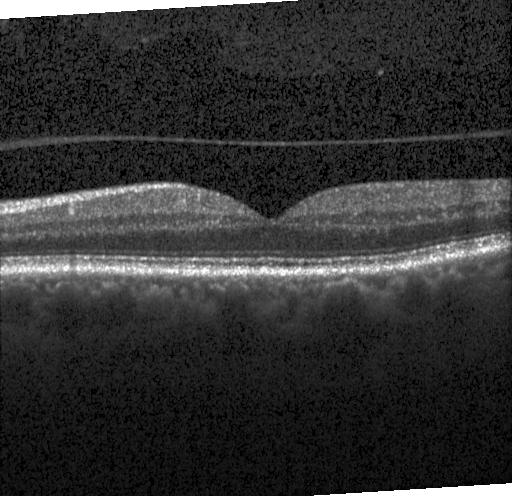

Instrument: Heidelberg Spectralis · macular scan · optical coherence tomography scan. Assessment: no evidence of choroidal neovascularization, diabetic macular edema, or drusen.